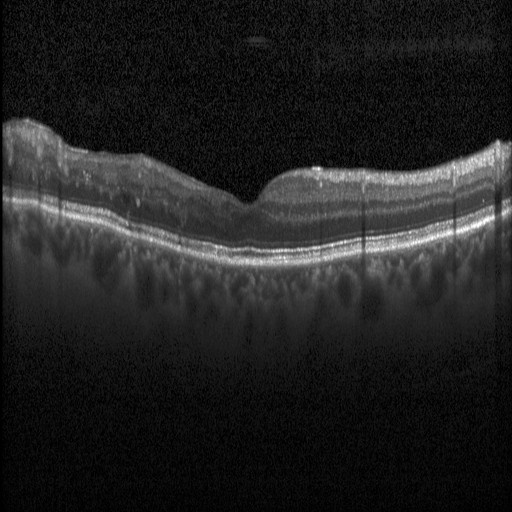 Retinal OCT B-scan — Finding: DME.